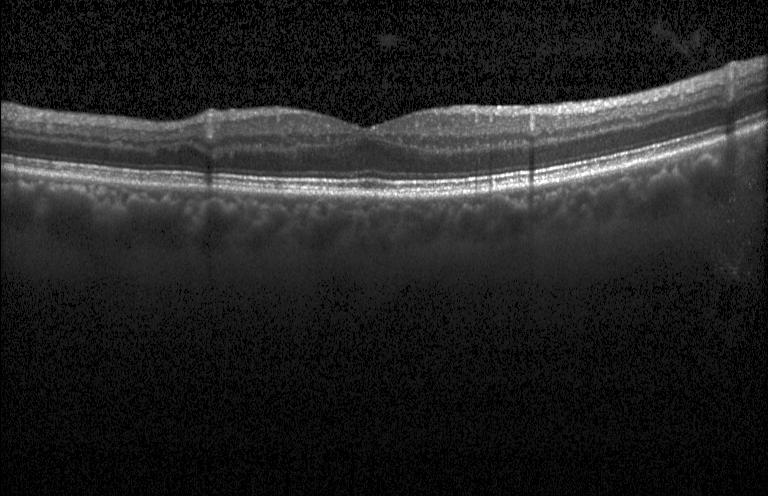
Assessment: no evidence of choroidal neovascularization, diabetic macular edema, or drusen.